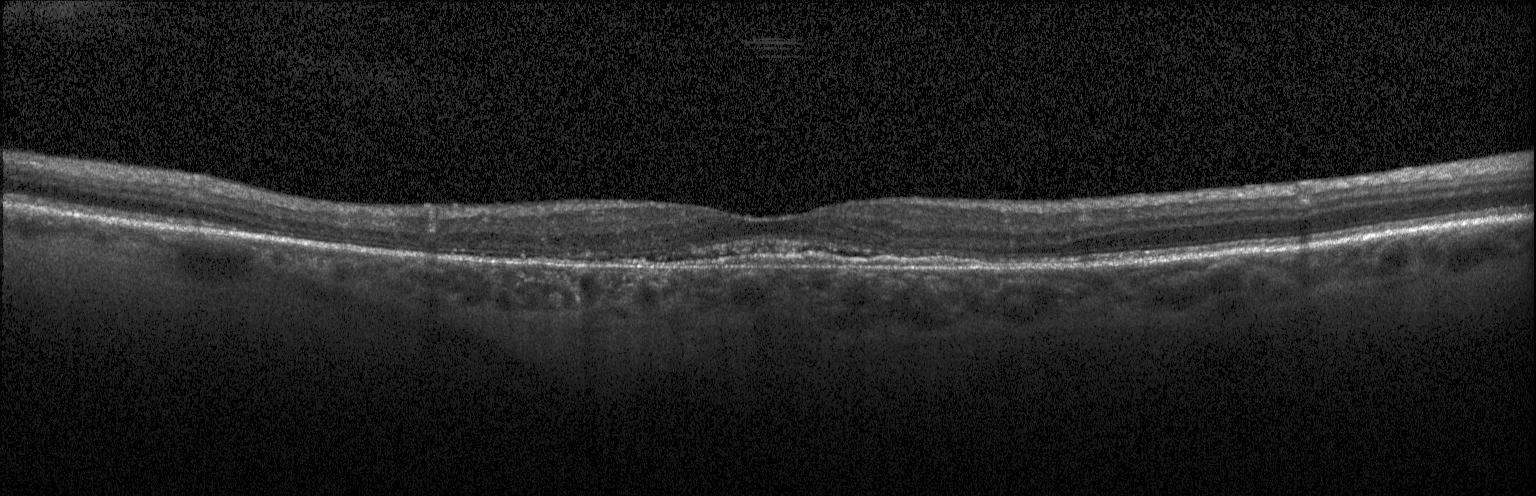

Heidelberg Spectralis. Fovea-centered. Retinal OCT cross-section
This B-scan demonstrates a choroidal neovascular membrane.